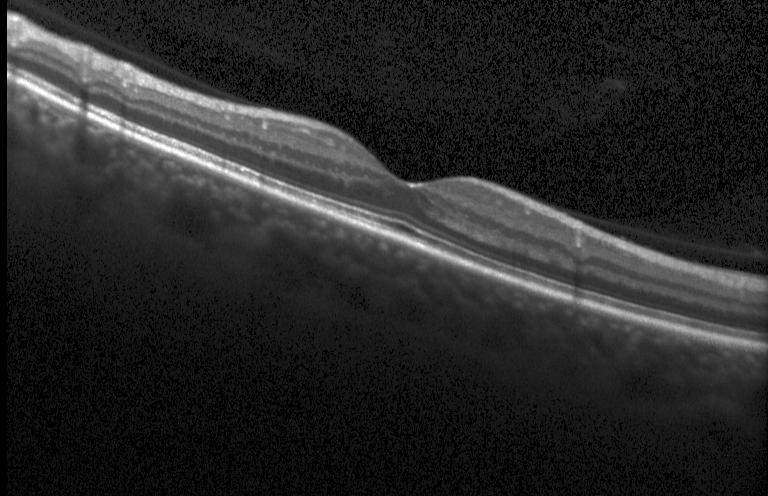 Finding: neither choroidal neovascularization, diabetic macular edema, nor drusen.